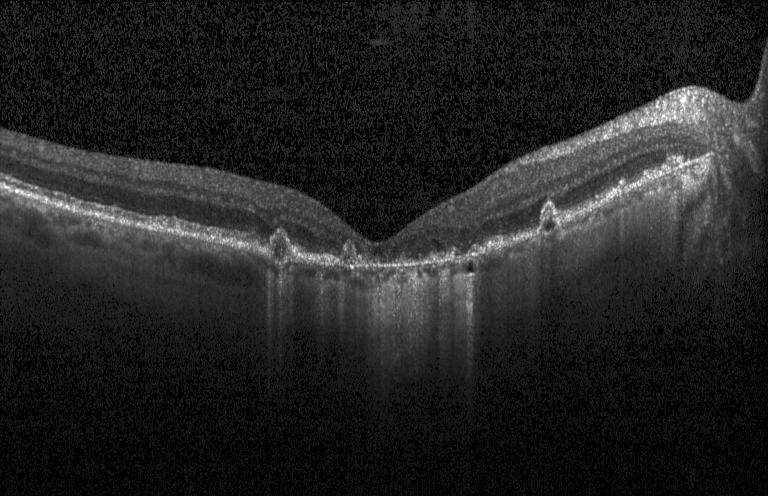

Diagnosis: CNV.